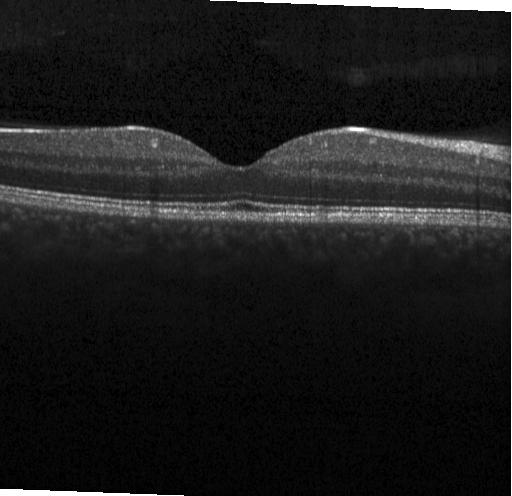

Spectral-domain optical coherence tomography. Retinal OCT cross-section. Centered on the fovea. Acquired on a Heidelberg Spectralis.
This B-scan demonstrates no CNV, no DME, and no drusen.